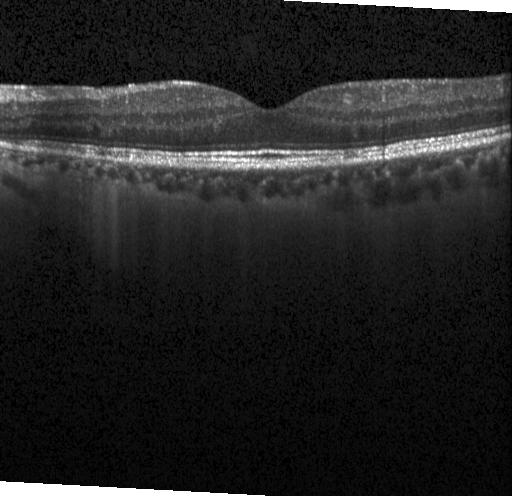

Fovea-centered; optical coherence tomography scan — Neither choroidal neovascularization, diabetic macular edema, nor drusen.